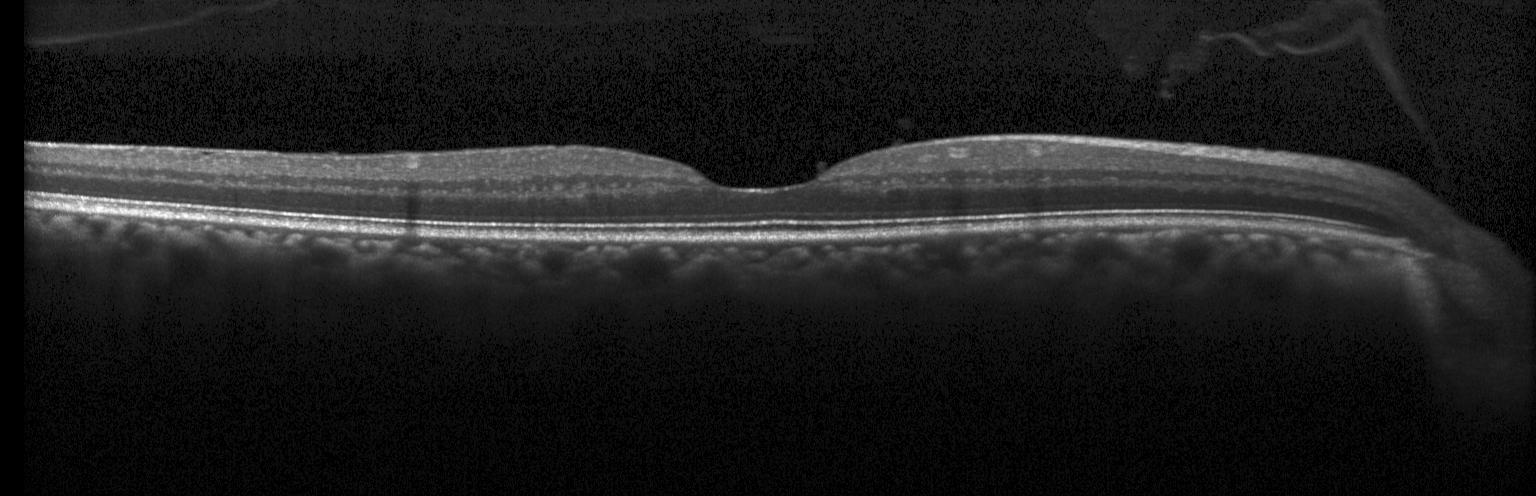

Dx: no choroidal neovascularization, diabetic macular edema, or drusen.